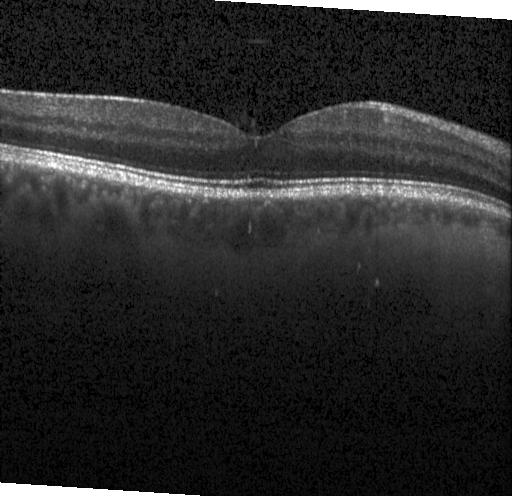
Centered on the fovea; retinal OCT cross-section; SD-OCT
Finding: neither CNV, DME, nor drusen.